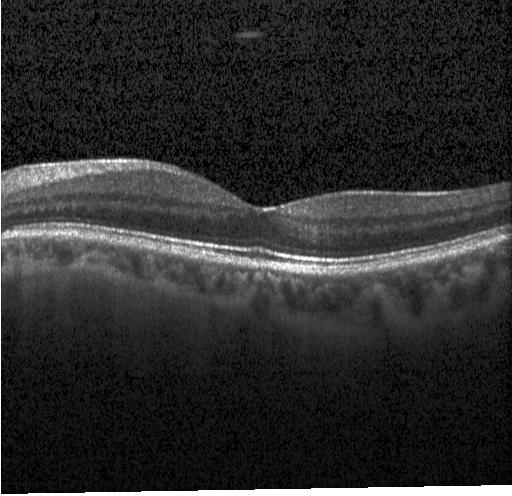

SD-OCT · retinal OCT B-scan · acquired on a Heidelberg Spectralis
Impression: no choroidal neovascularization, diabetic macular edema, or drusen.